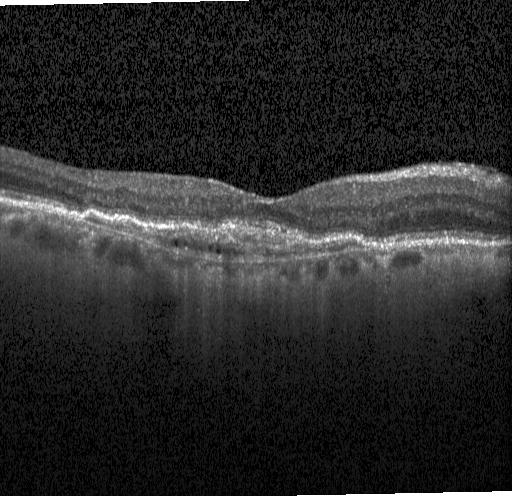
Diagnosis: a choroidal neovascular membrane.